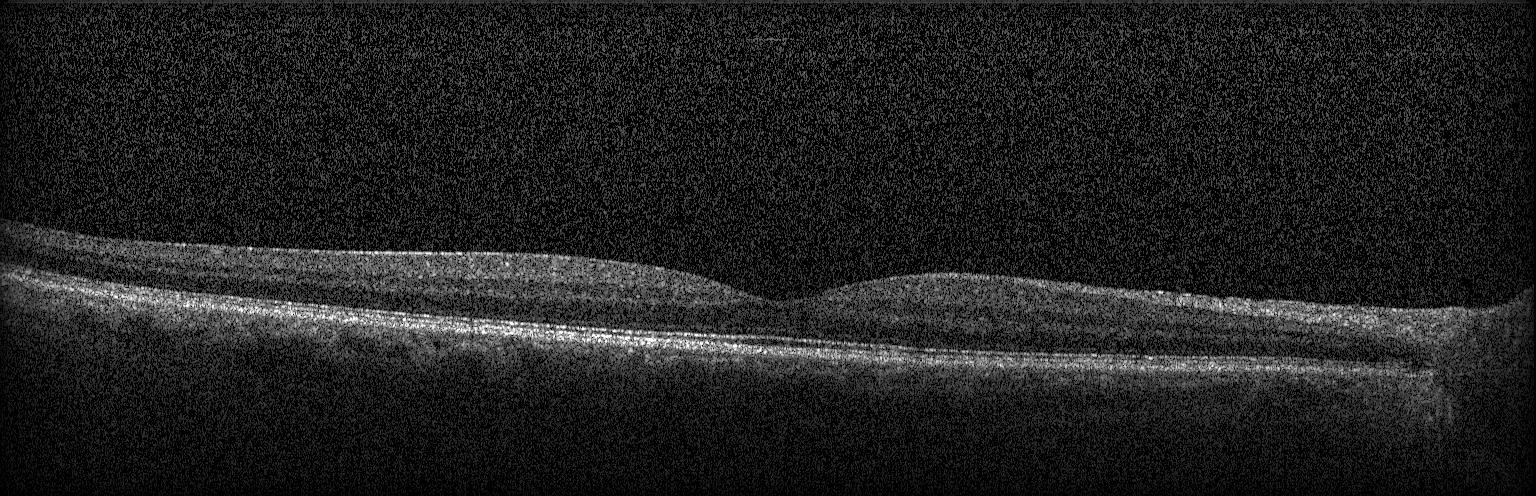

Spectral-domain OCT B-scan: neither CNV, DME, nor drusen.